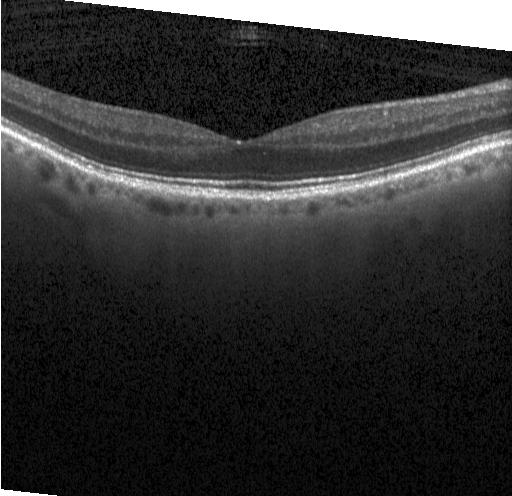

SD-OCT. Heidelberg Spectralis. Optical coherence tomography scan.
No evidence of CNV, DME, or drusen.